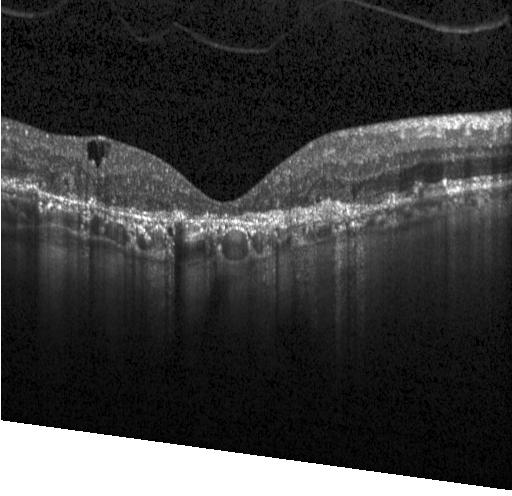

Impression: a choroidal neovascular membrane.